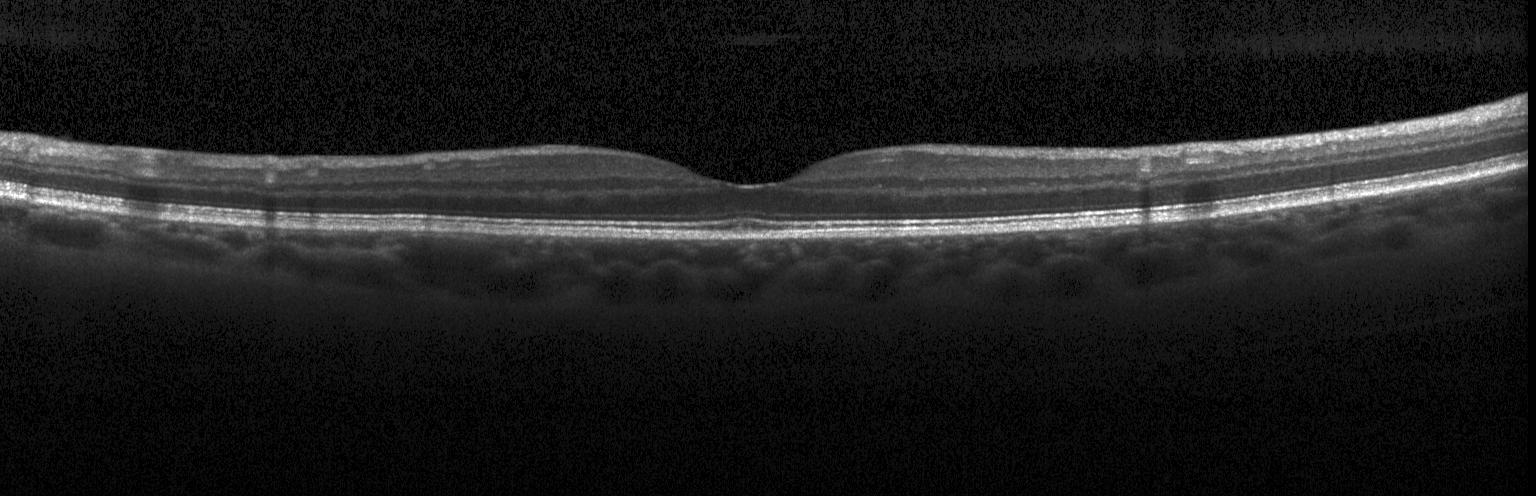 Retinal OCT B-scan; acquired on a Heidelberg Spectralis
Finding: no evidence of CNV, DME, or drusen.